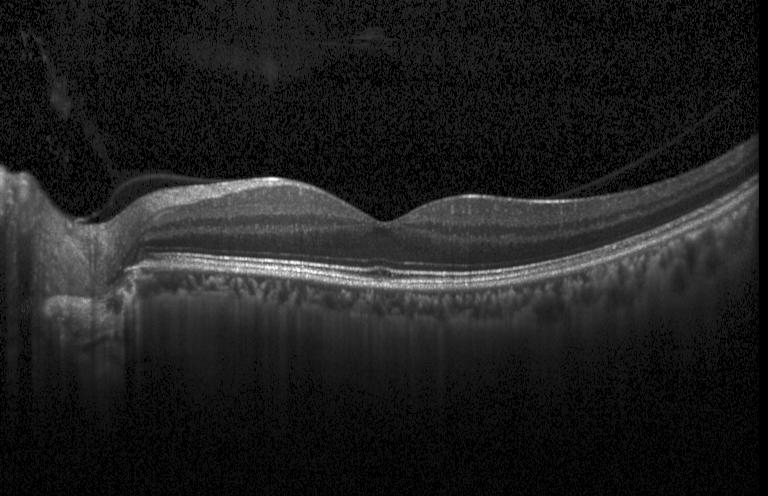

Impression: no CNV, no DME, and no drusen.